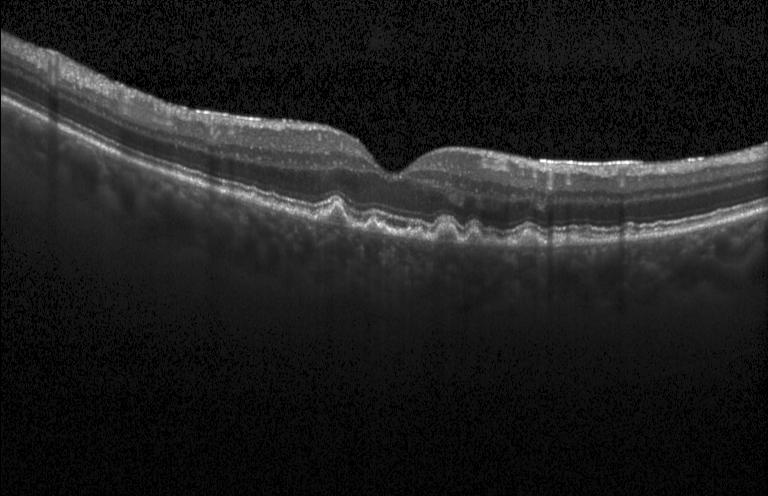 Retinal OCT B-scan. Assessment: sub-RPE drusenoid deposits.